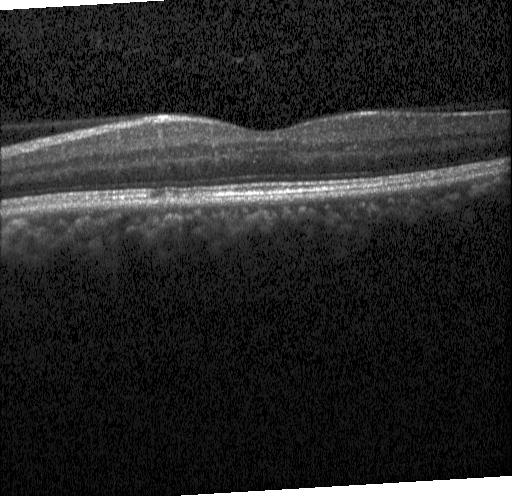 OCT scan showing no evidence of choroidal neovascularization, diabetic macular edema, or drusen.